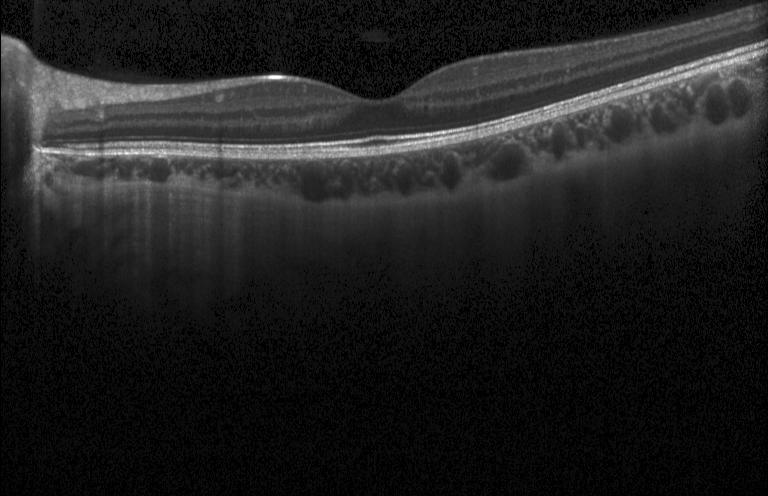

Spectral-domain OCT B-scan: no CNV, DME, or drusen.